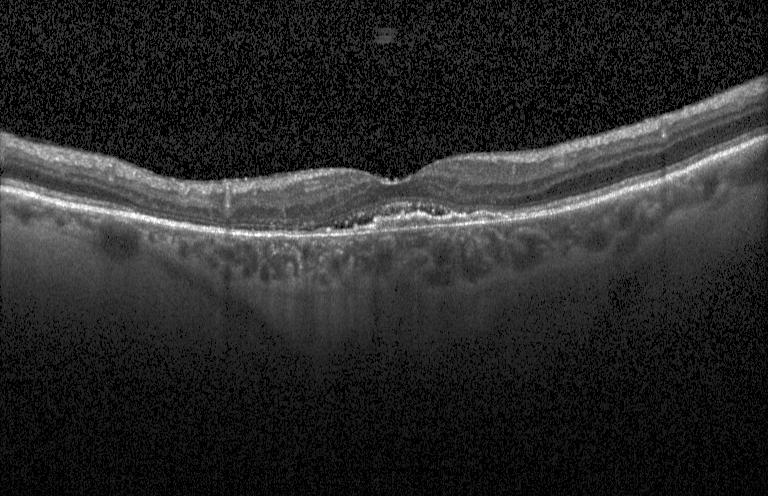

Centered on the fovea · OCT line scan.
Impression: a choroidal neovascular membrane.